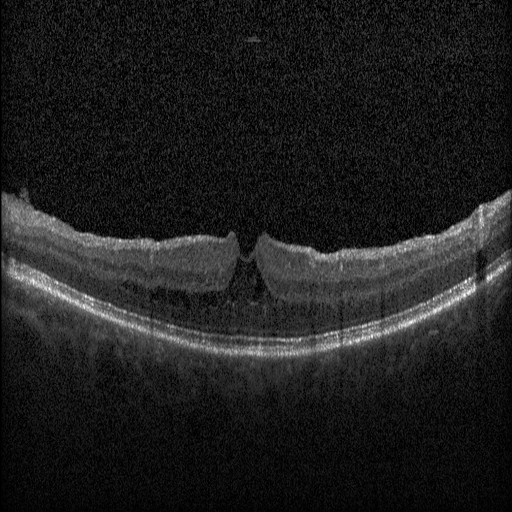
OCT B-scan.
Finding: diabetic macular edema (DME).